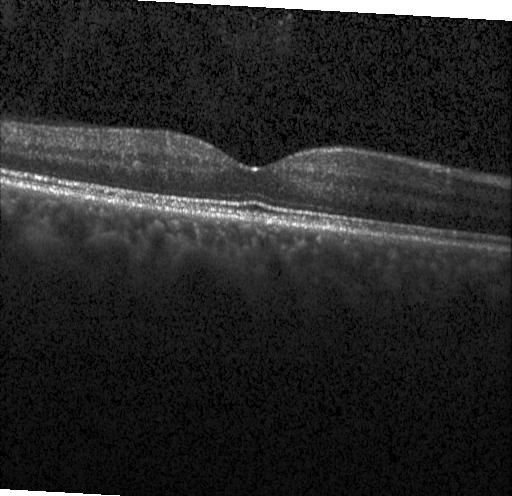 OCT B-scan showing no choroidal neovascularization, no diabetic macular edema, and no drusen.